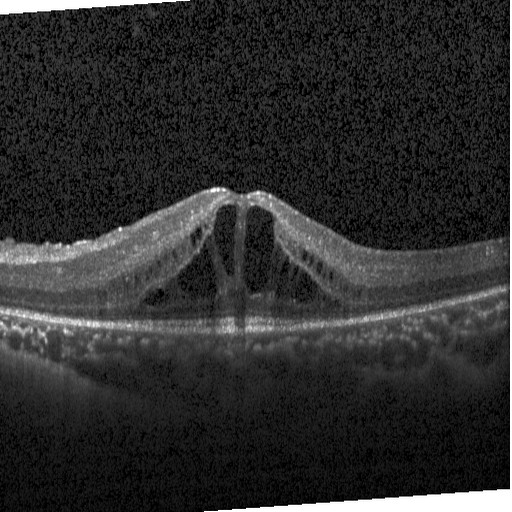
Dx: DME.